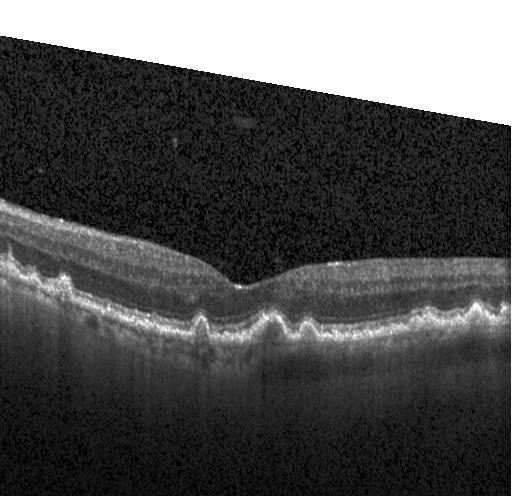 Assessment: sub-RPE drusenoid deposits.